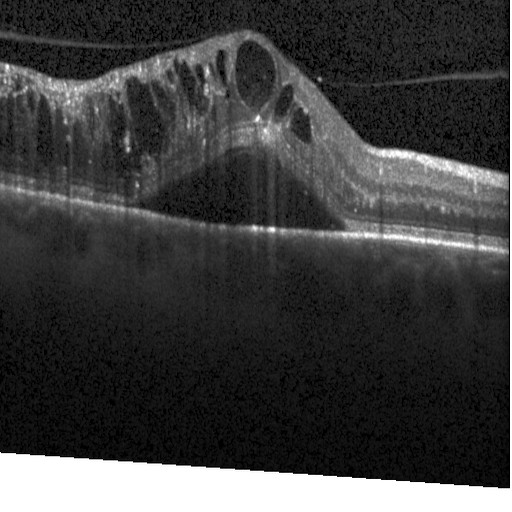 Retinal OCT B-scan, spectral-domain optical coherence tomography, through the macula — Finding: diabetic macular edema.